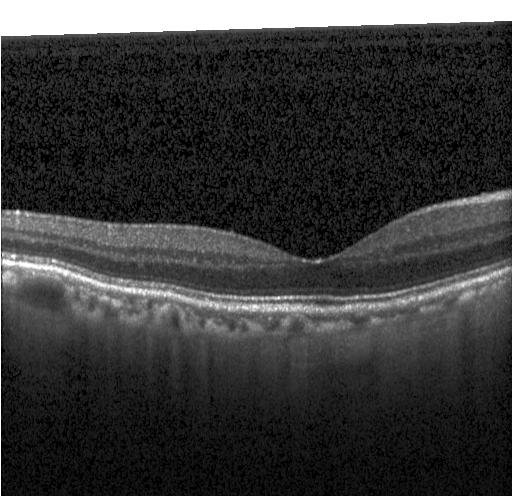
Heidelberg Spectralis. OCT B-scan. SD-OCT. This B-scan demonstrates no choroidal neovascularization, diabetic macular edema, or drusen.